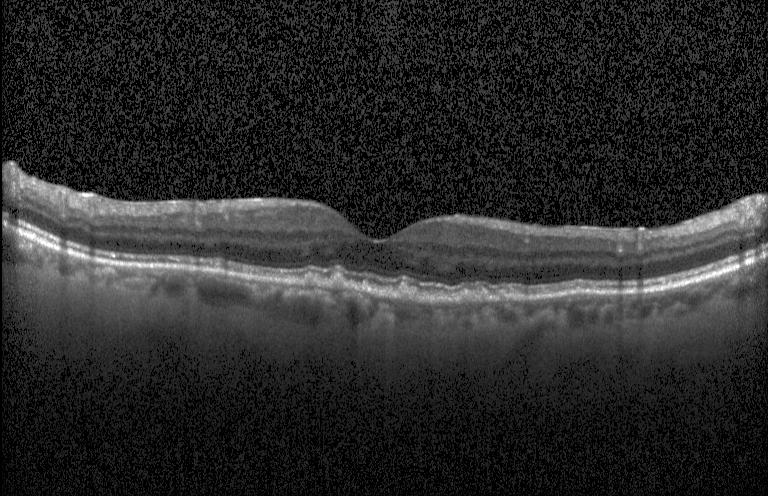

Optical coherence tomography scan; spectral-domain OCT; instrument: Heidelberg Spectralis; horizontal scan through the fovea — Diagnosis: multiple drusen.